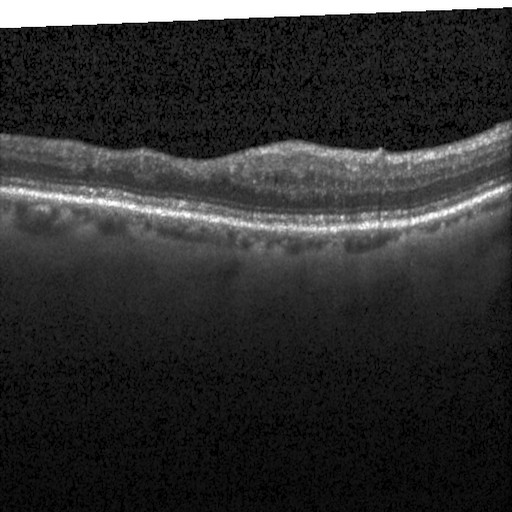 Spectral-domain optical coherence tomography, optical coherence tomography B-scan, macular scan, Heidelberg Spectralis — Diagnosis: DME.